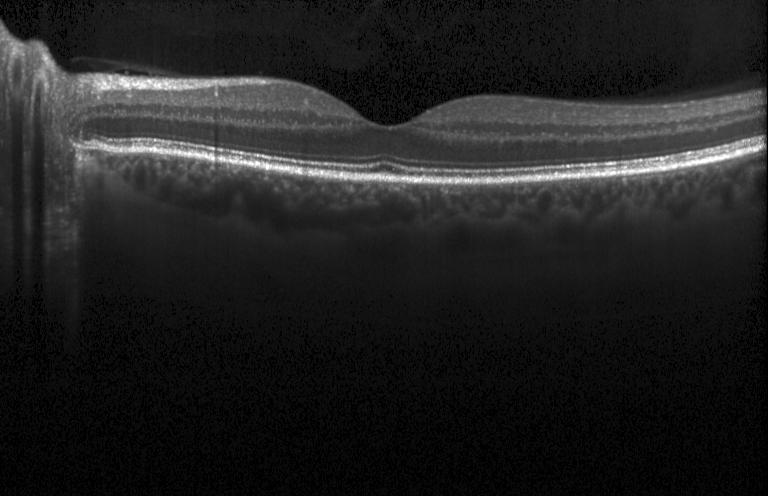 Finding: no evidence of CNV, DME, or drusen.